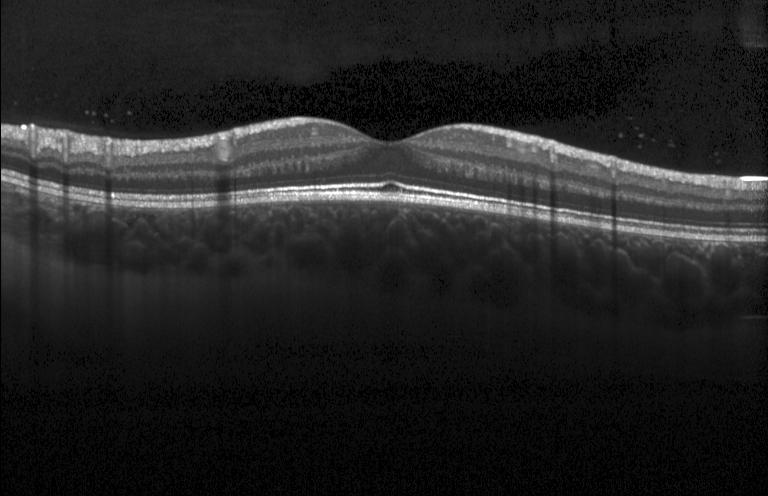

This B-scan demonstrates no evidence of choroidal neovascularization, diabetic macular edema, or drusen.